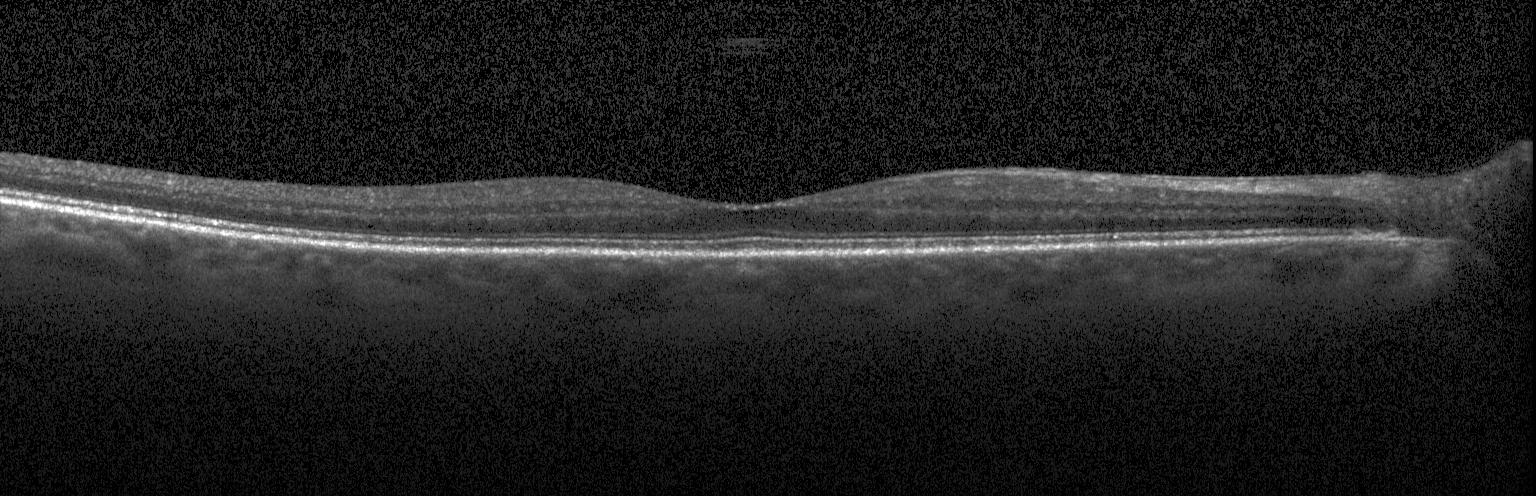
Acquired on a Heidelberg Spectralis · OCT B-scan · SD-OCT · centered on the fovea.
This B-scan demonstrates neither choroidal neovascularization, diabetic macular edema, nor drusen.